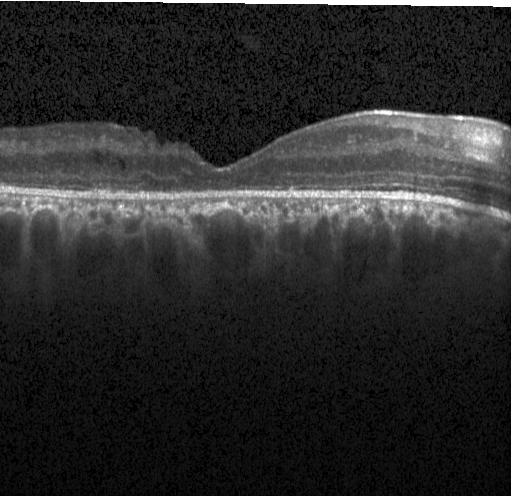

Through the macula, retinal OCT cross-section. The scan shows diabetic macular edema (DME).